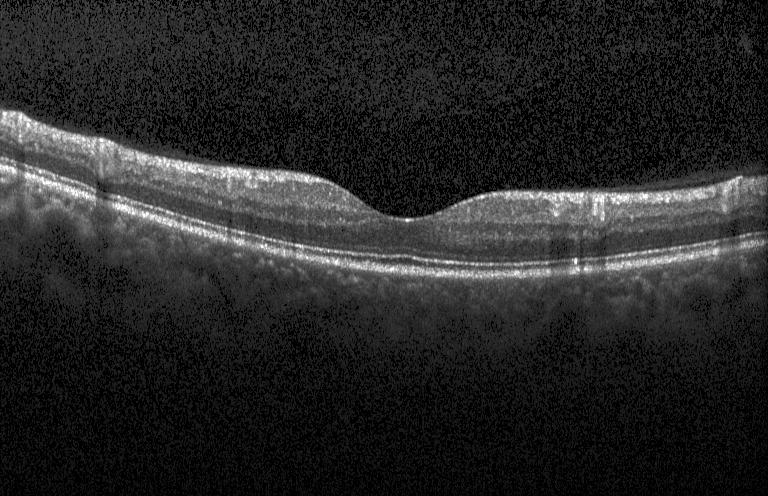

Finding: neither choroidal neovascularization, diabetic macular edema, nor drusen.